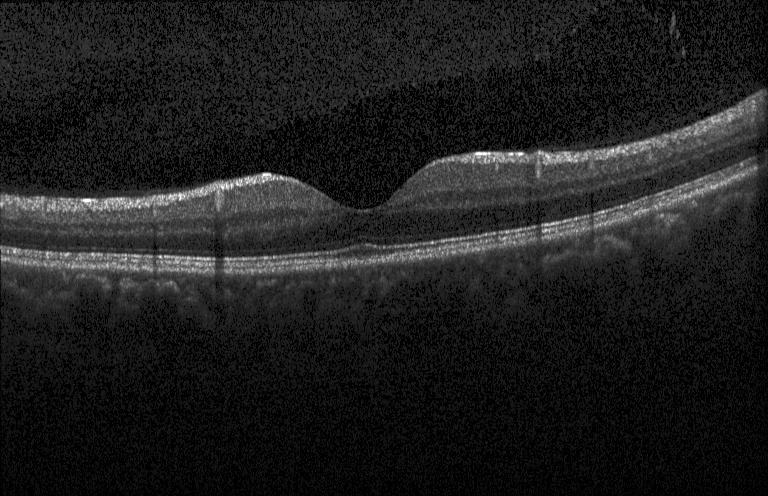

Optical coherence tomography B-scan · through the macula · spectral-domain OCT · acquired on a Heidelberg Spectralis — Finding: neither CNV, DME, nor drusen.